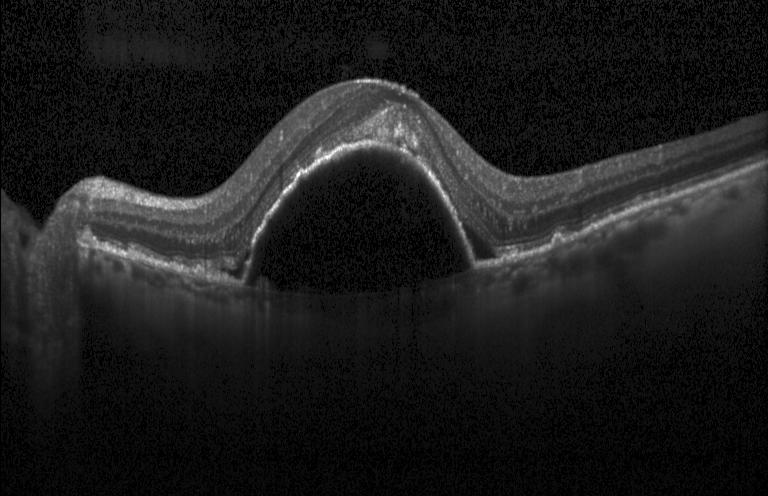

Retinal OCT cross-section · spectral-domain OCT.
Impression: choroidal neovascularization.